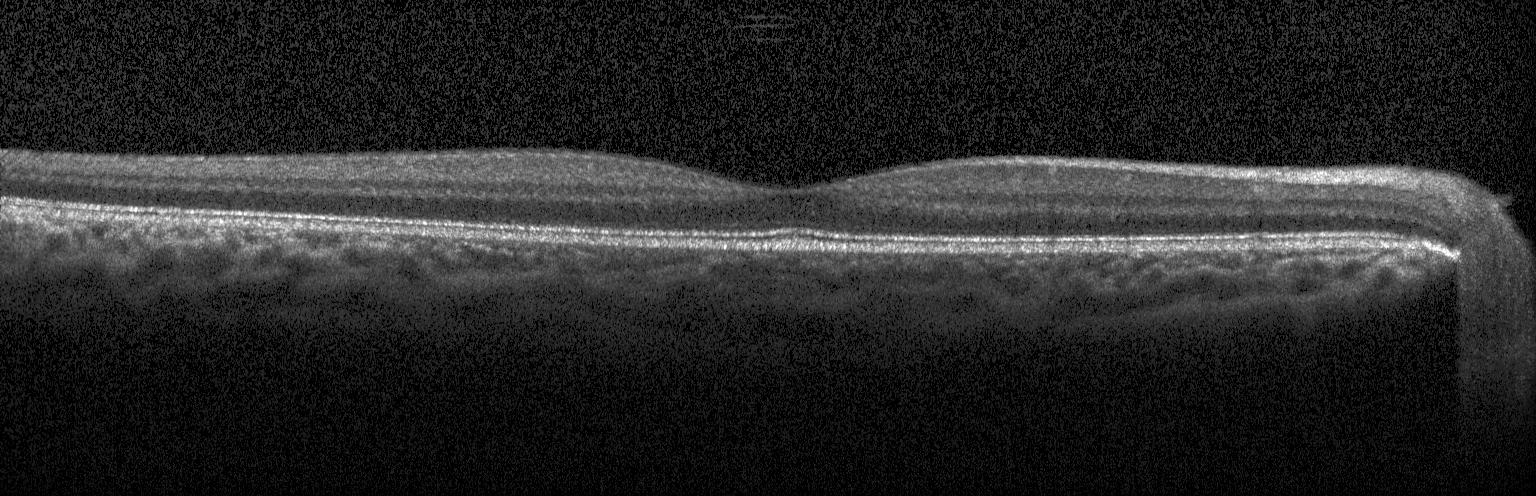 OCT B-scan, spectral-domain OCT
Diagnosis: neither CNV, DME, nor drusen.